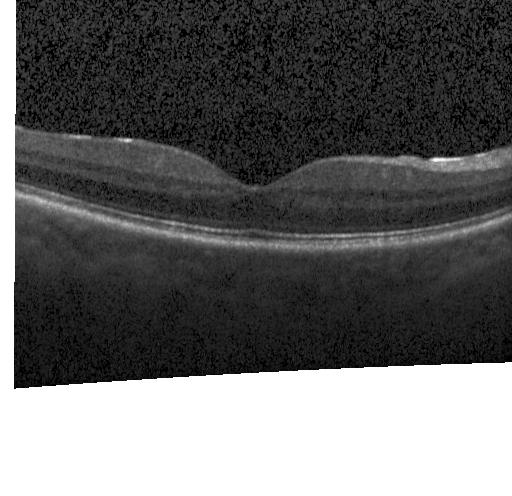

Retinal OCT B-scan
No evidence of CNV, DME, or drusen.